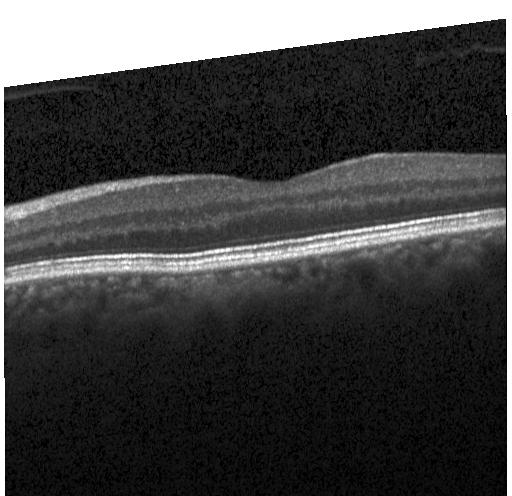 Retinal OCT cross-section · spectral-domain optical coherence tomography · Heidelberg Spectralis OCT system. Finding: no choroidal neovascularization, no diabetic macular edema, and no drusen.